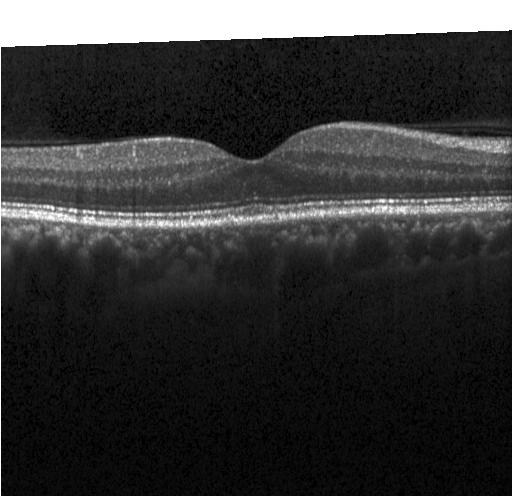 Macular OCT: no evidence of choroidal neovascularization, diabetic macular edema, or drusen.